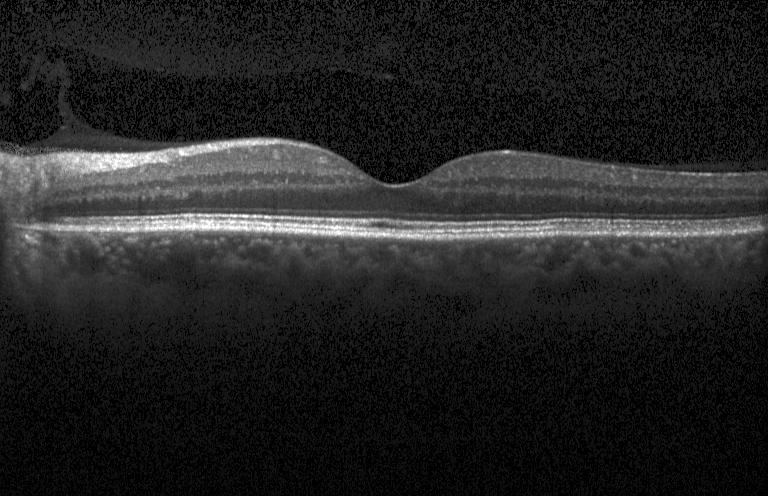

Retinal OCT B-scan. No evidence of CNV, DME, or drusen.